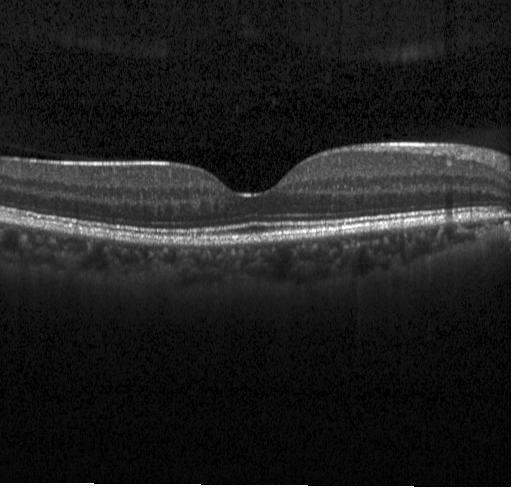
Fovea-centered · optical coherence tomography B-scan · Heidelberg Spectralis OCT system. Impression: neither choroidal neovascularization, diabetic macular edema, nor drusen.